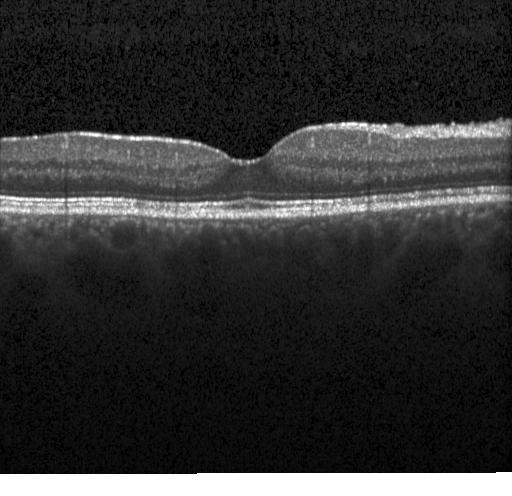
Heidelberg Spectralis; macular scan; optical coherence tomography scan — Impression: neither choroidal neovascularization, diabetic macular edema, nor drusen.